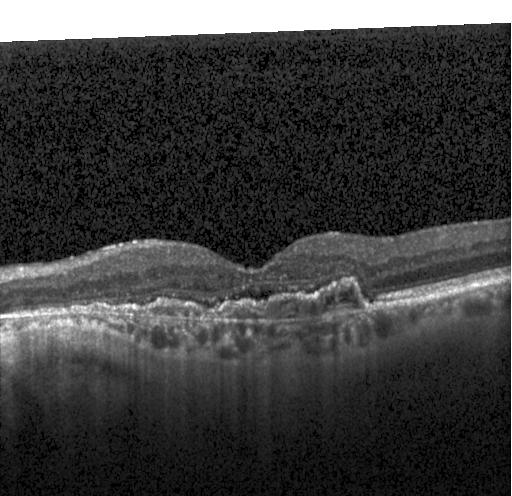 Spectral-domain optical coherence tomography, retinal OCT B-scan. Impression: choroidal neovascularization (CNV).